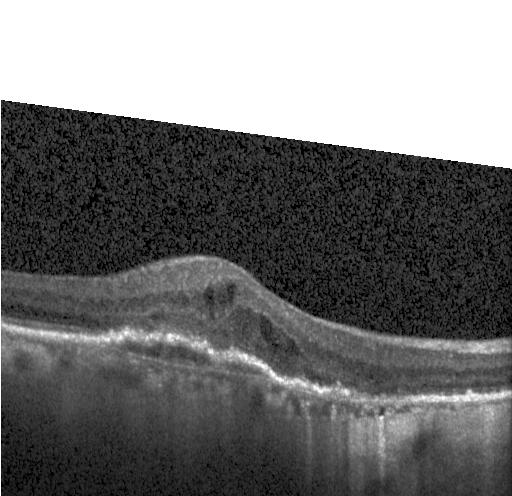 Finding: a choroidal neovascular membrane.